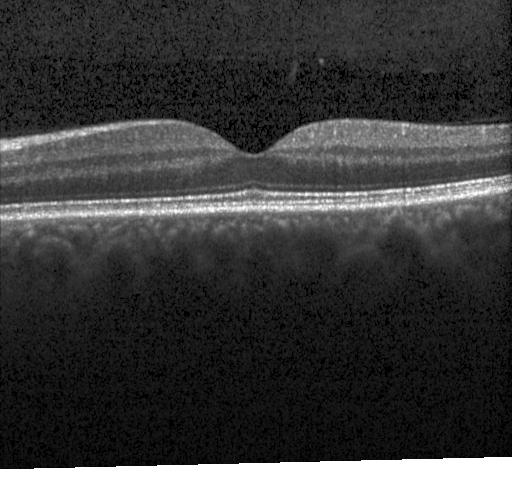 Heidelberg Spectralis. OCT B-scan. Fovea-centered — Macular OCT: neither choroidal neovascularization, diabetic macular edema, nor drusen.